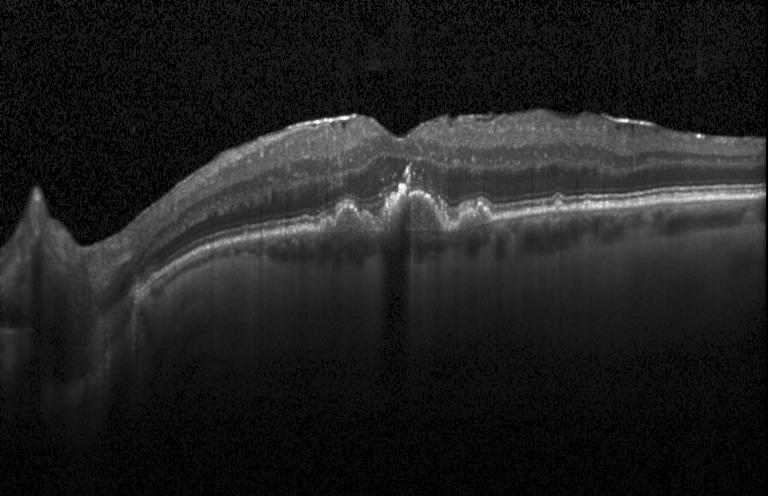

Optical coherence tomography scan
Dx: multiple drusen.